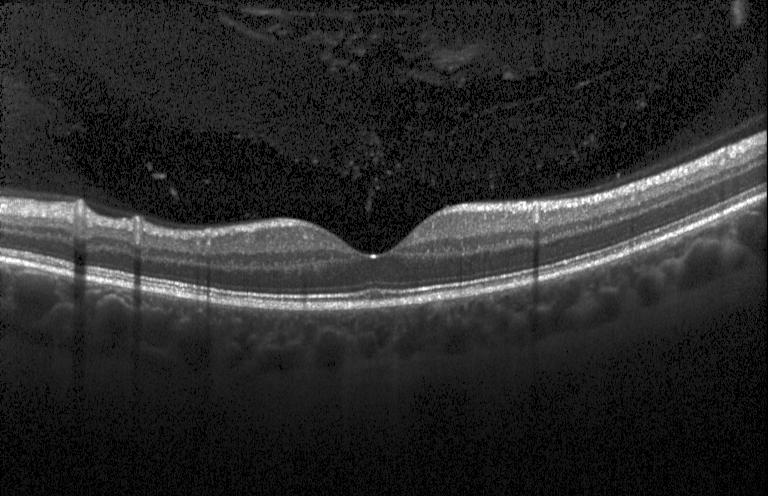
OCT line scan
Macular OCT: no evidence of CNV, DME, or drusen.